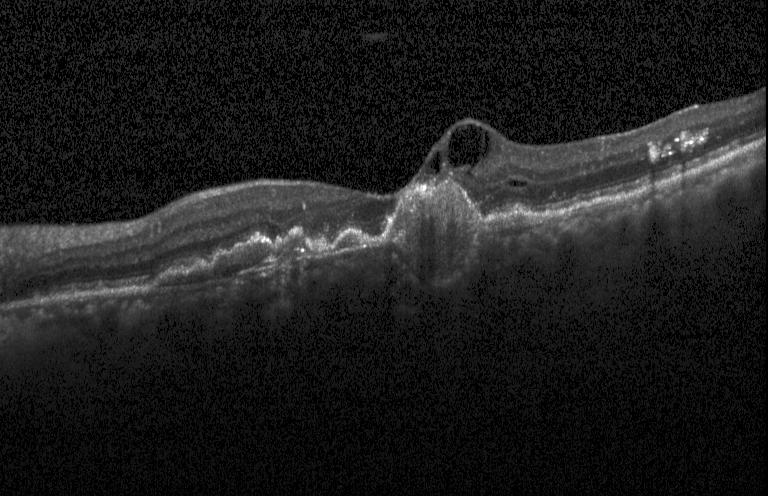 Retinal OCT cross-section, centered on the fovea.
The scan shows CNV.